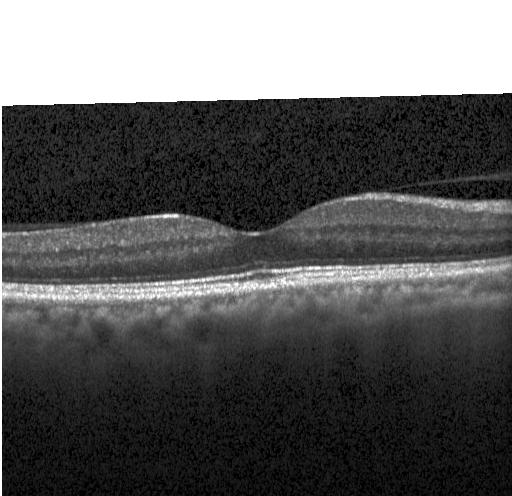

Heidelberg Spectralis OCT system · OCT line scan.
The scan shows no CNV, DME, or drusen.